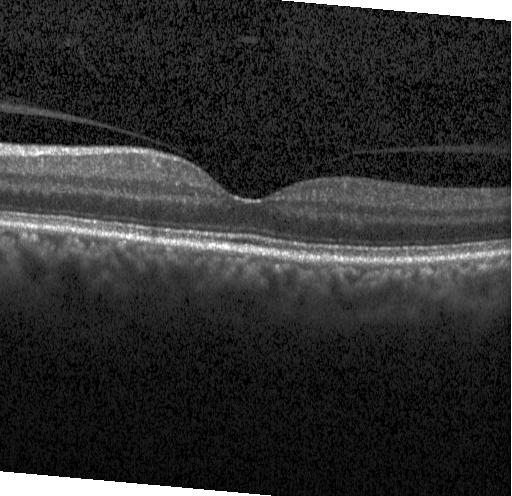
OCT B-scan, instrument: Heidelberg Spectralis, horizontal scan through the fovea — Impression: no CNV, no DME, and no drusen.